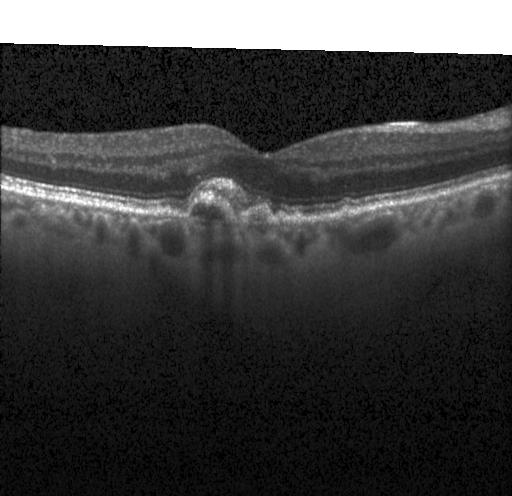
OCT B-scan
Impression: a choroidal neovascular membrane.